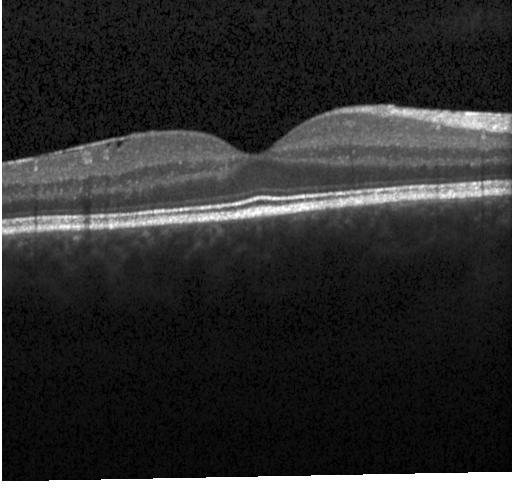
The scan shows neither choroidal neovascularization, diabetic macular edema, nor drusen.